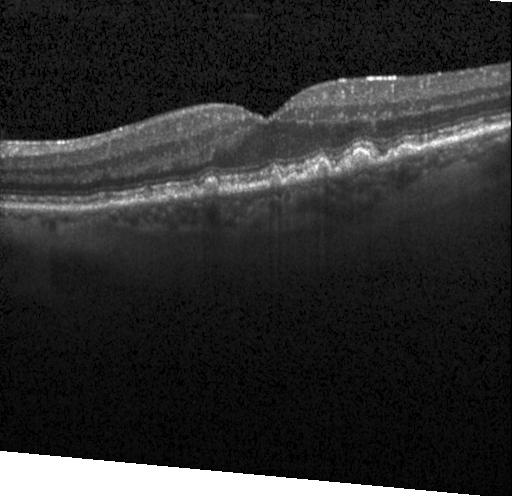
Assessment: drusen.